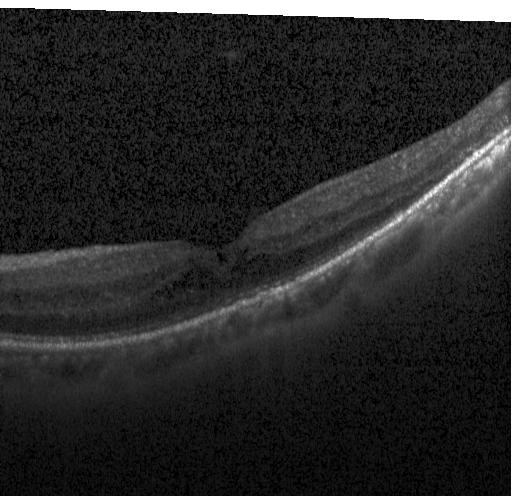

Finding: diabetic macular edema (DME).